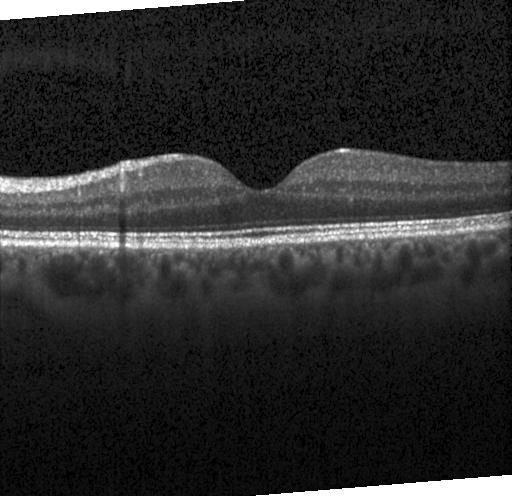
Spectral-domain OCT. Retinal OCT cross-section — This B-scan demonstrates neither CNV, DME, nor drusen.